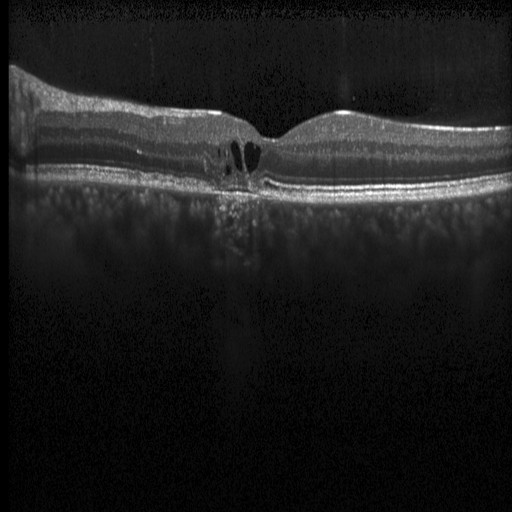
Heidelberg Spectralis, spectral-domain OCT, OCT B-scan, macular scan.
This B-scan demonstrates DME.